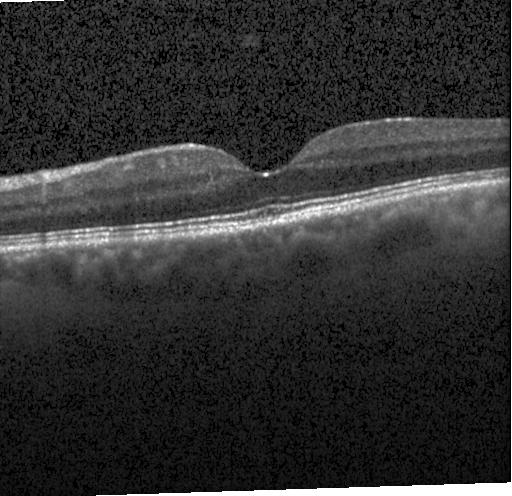

Optical coherence tomography B-scan. This B-scan demonstrates neither choroidal neovascularization, diabetic macular edema, nor drusen.